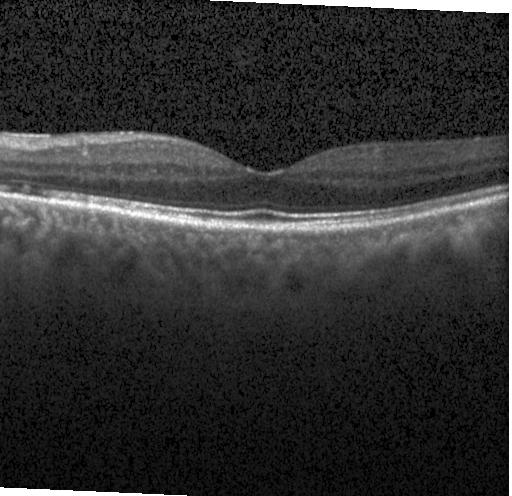

Impression: no choroidal neovascularization, no diabetic macular edema, and no drusen.